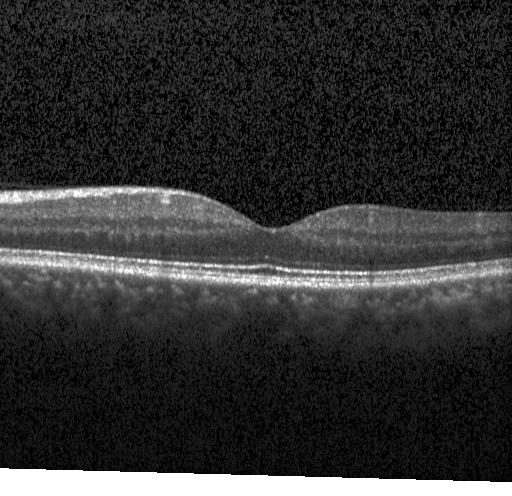
Retinal OCT B-scan. SD-OCT.
No choroidal neovascularization, diabetic macular edema, or drusen.